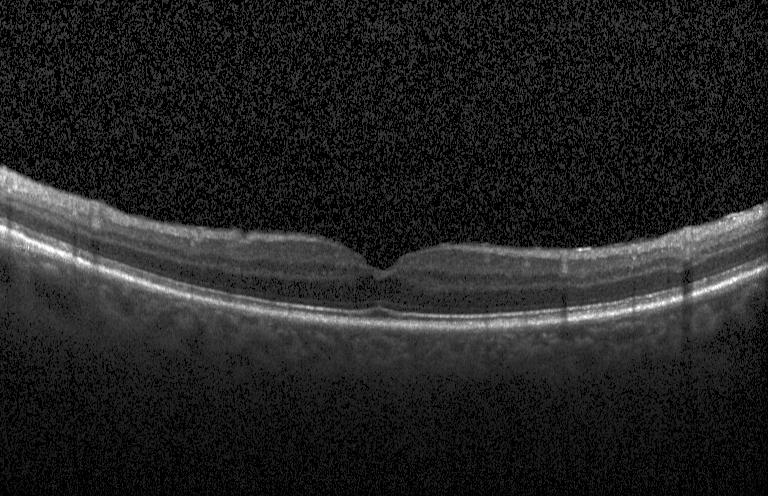

Spectral-domain OCT. Through the macula. Optical coherence tomography B-scan. Diagnosis: neither choroidal neovascularization, diabetic macular edema, nor drusen.